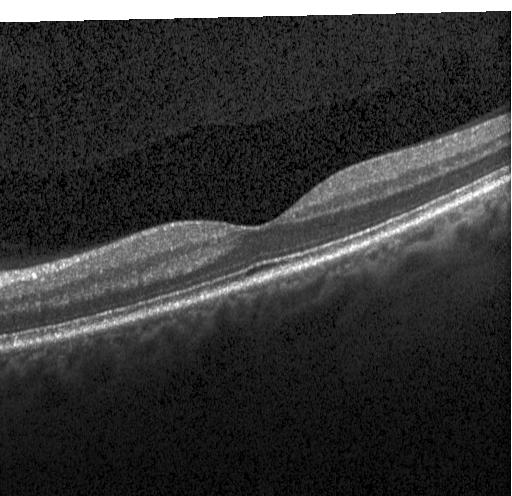

Heidelberg Spectralis; horizontal scan through the fovea; optical coherence tomography B-scan. No evidence of choroidal neovascularization, diabetic macular edema, or drusen.